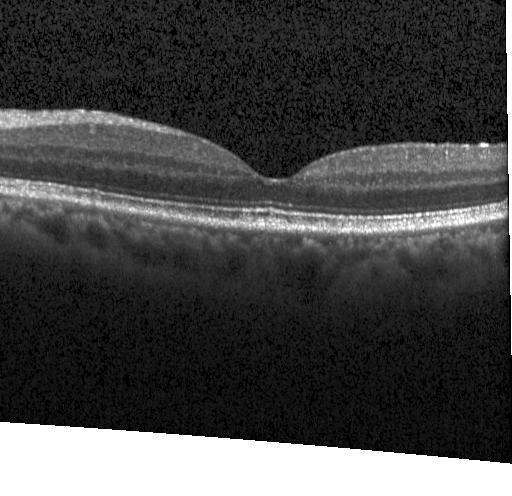 This B-scan demonstrates no evidence of CNV, DME, or drusen.